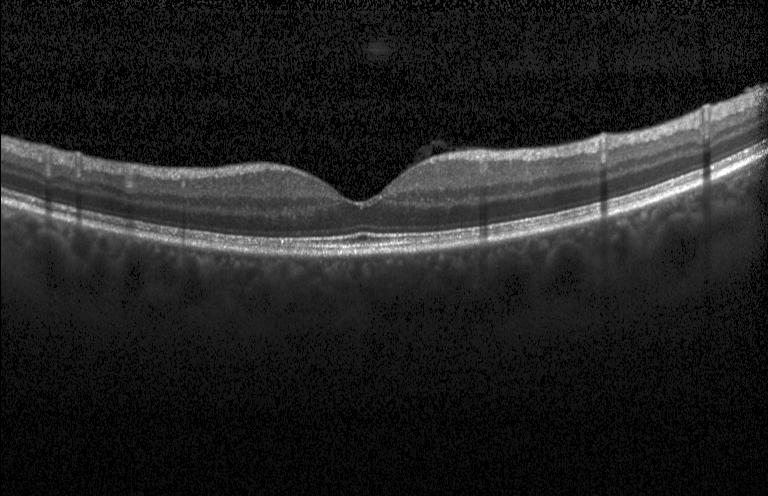

Heidelberg Spectralis OCT system; OCT B-scan; macular scan — Dx: no evidence of choroidal neovascularization, diabetic macular edema, or drusen.